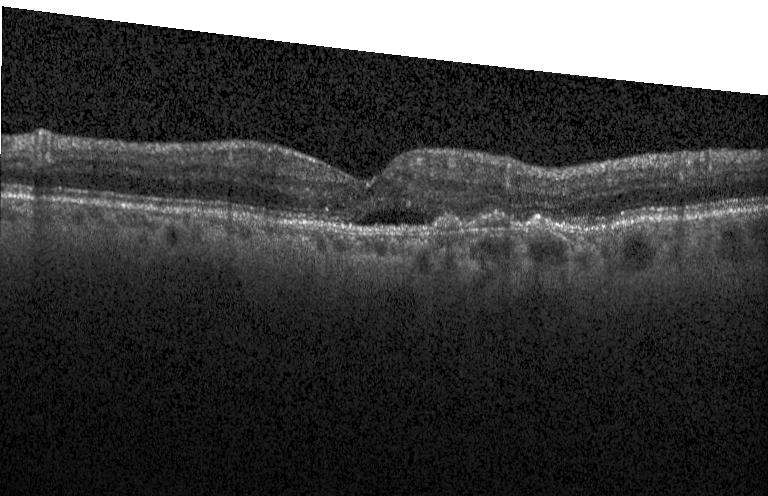

Spectral-domain OCT B-scan: a choroidal neovascular membrane.